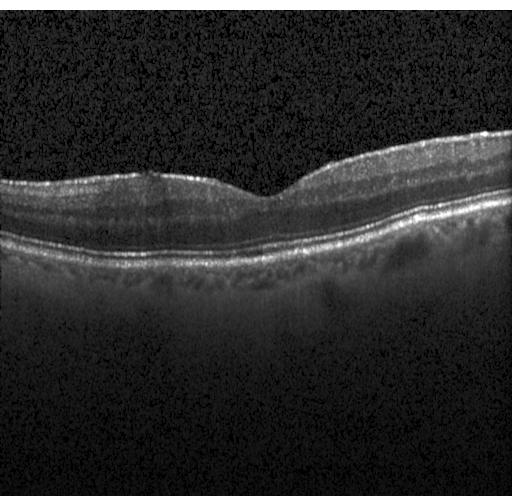

Diagnosis: neither choroidal neovascularization, diabetic macular edema, nor drusen.